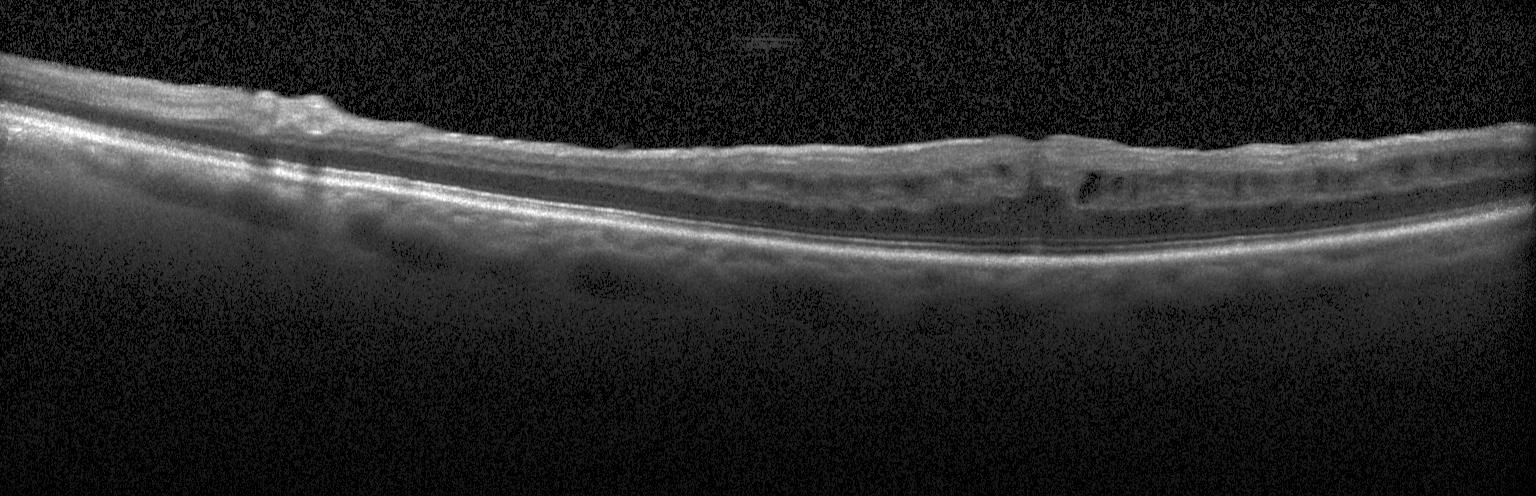 The scan shows DME.